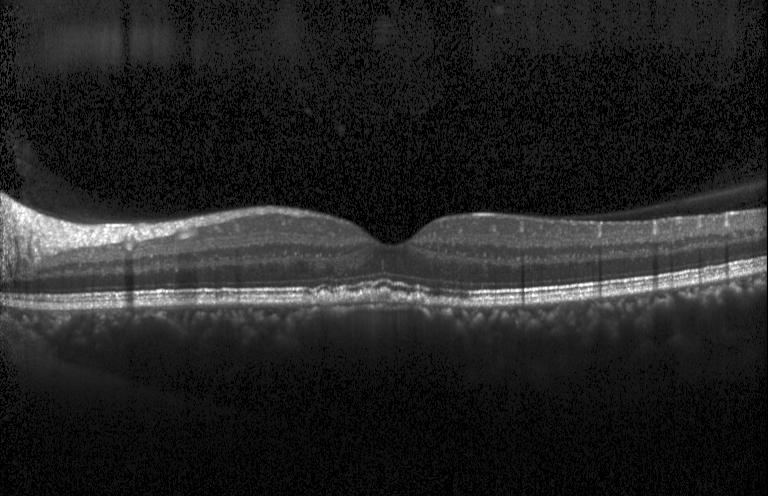 Centered on the fovea. Optical coherence tomography B-scan
Assessment: drusen.